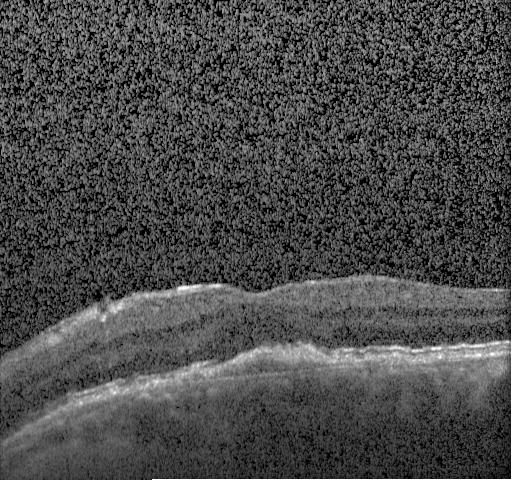
OCT scan showing choroidal neovascularization.